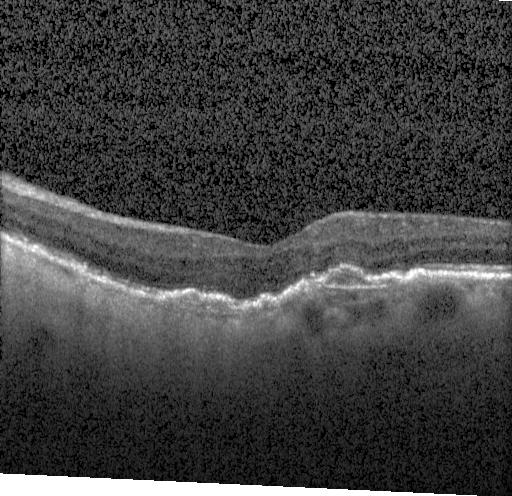 Impression: a choroidal neovascular membrane.